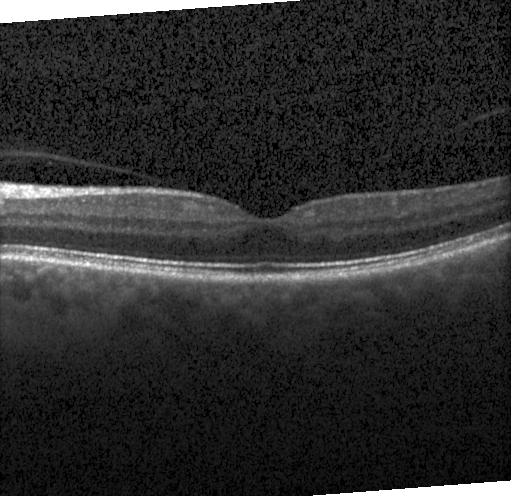 Heidelberg Spectralis OCT system; OCT line scan. Assessment: no choroidal neovascularization, no diabetic macular edema, and no drusen.